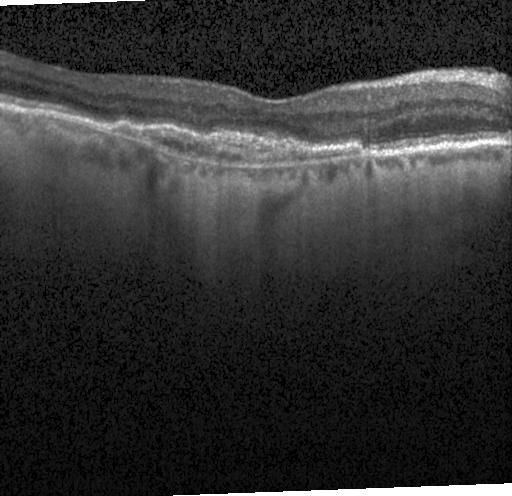
Optical coherence tomography B-scan
Diagnosis: a choroidal neovascular membrane.